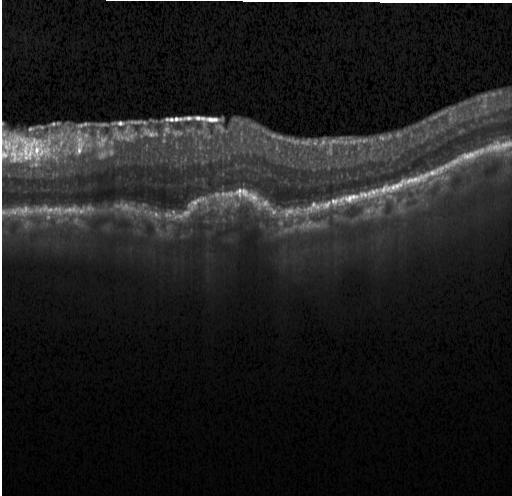
Through the macula, optical coherence tomography B-scan, spectral-domain OCT — Dx: choroidal neovascularization (CNV).